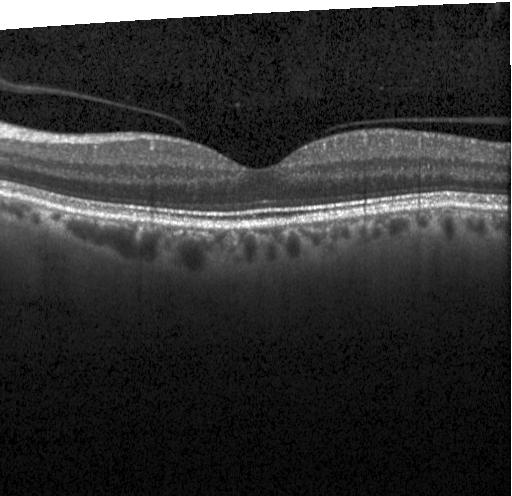
The scan shows neither CNV, DME, nor drusen.